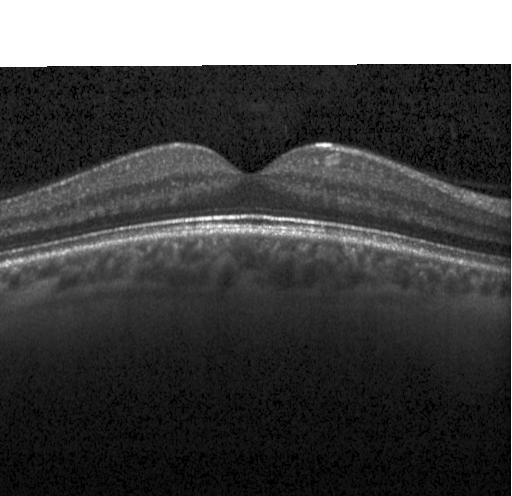

Optical coherence tomography scan; spectral-domain optical coherence tomography; through the macula.
Assessment: no choroidal neovascularization, diabetic macular edema, or drusen.